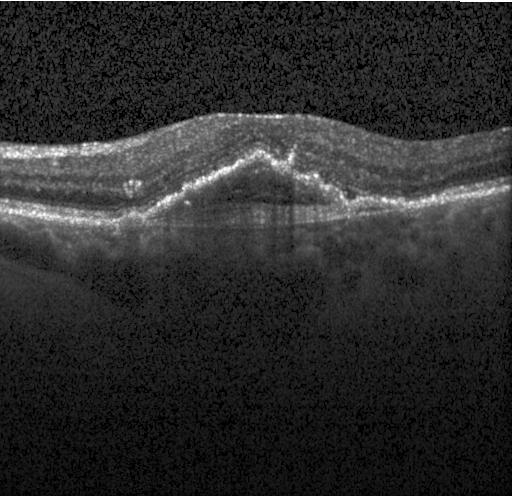 Retinal OCT cross-section · Heidelberg Spectralis OCT system · SD-OCT — A choroidal neovascular membrane.